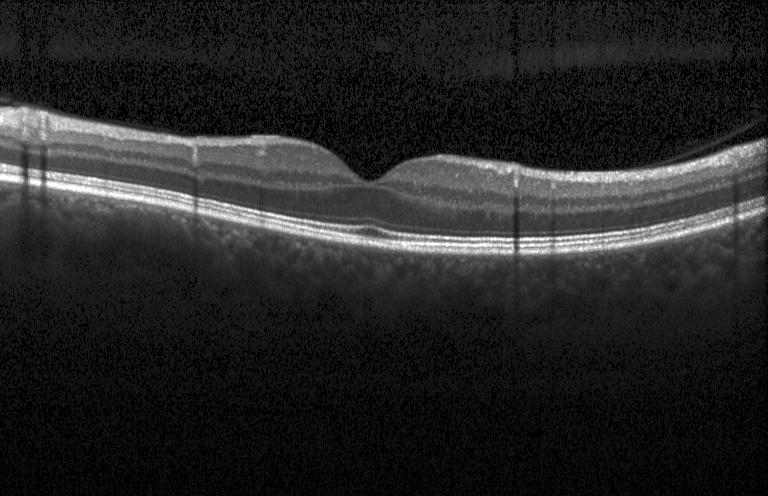 Optical coherence tomography scan; through the macula; SD-OCT. Macular OCT: no CNV, no DME, and no drusen.